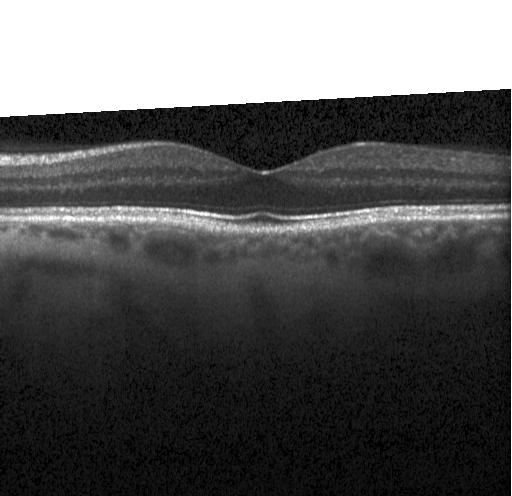
Heidelberg Spectralis OCT system · OCT line scan. OCT finding: neither CNV, DME, nor drusen.